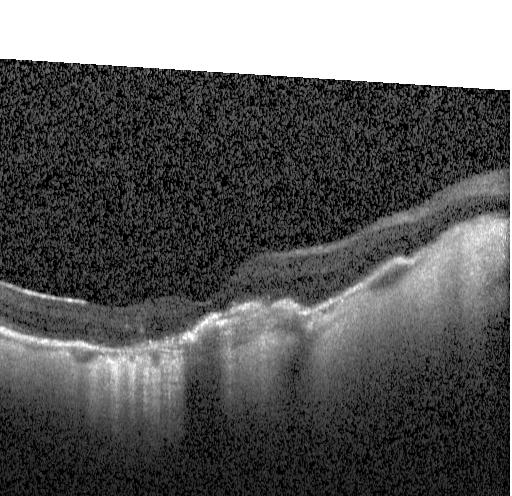
OCT B-scan. Spectral-domain OCT. Dx: choroidal neovascularization (CNV).